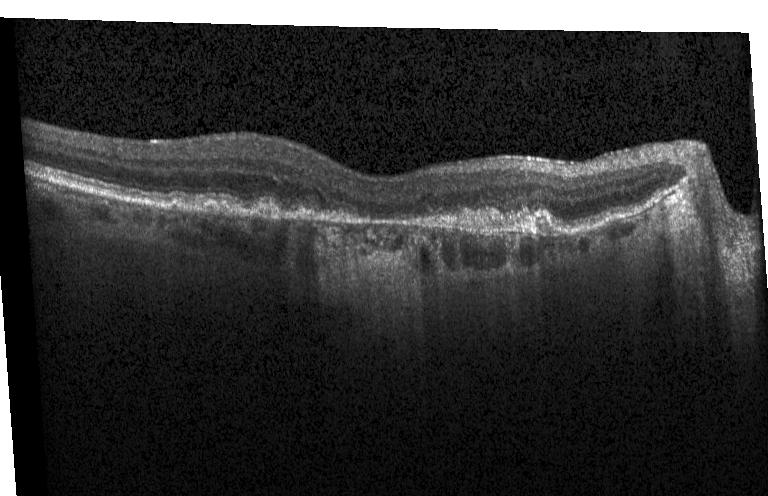 Heidelberg Spectralis · retinal OCT cross-section · horizontal scan through the fovea · SD-OCT
A choroidal neovascular membrane.